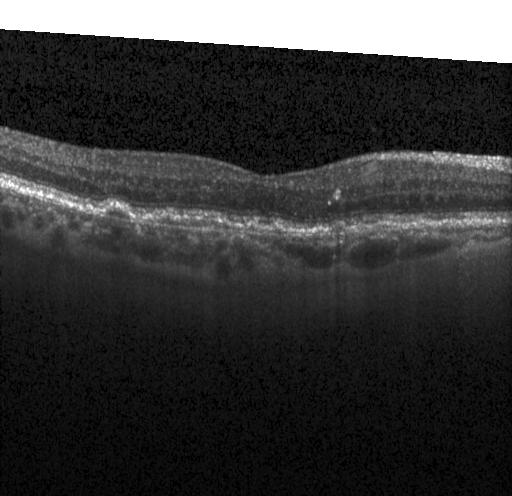
Finding: a choroidal neovascular membrane.